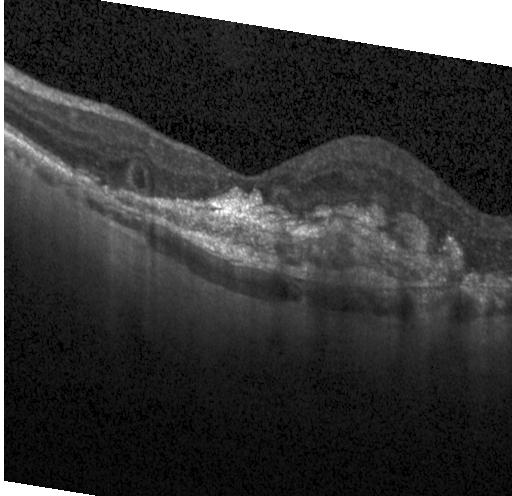

Dx: a choroidal neovascular membrane.